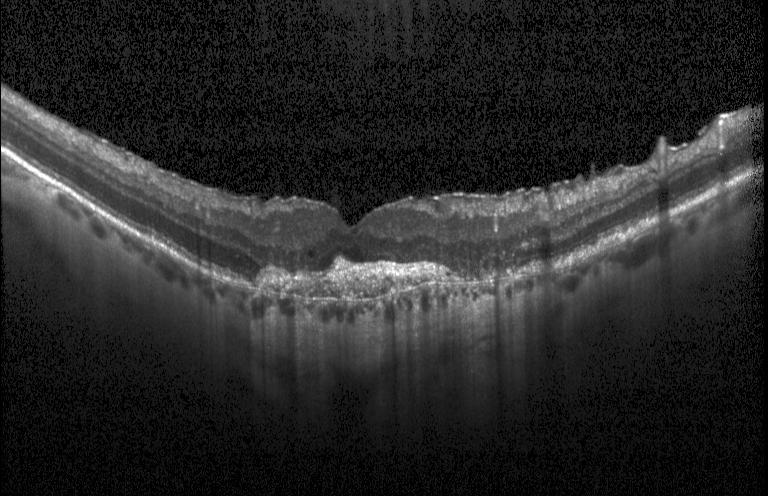

A choroidal neovascular membrane.